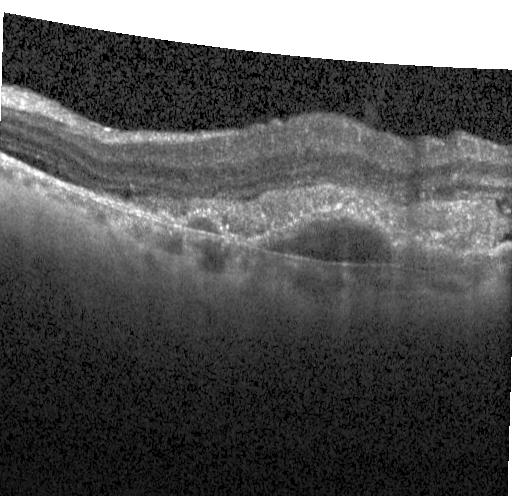 Through the macula. SD-OCT. OCT line scan.
OCT finding: choroidal neovascularization.